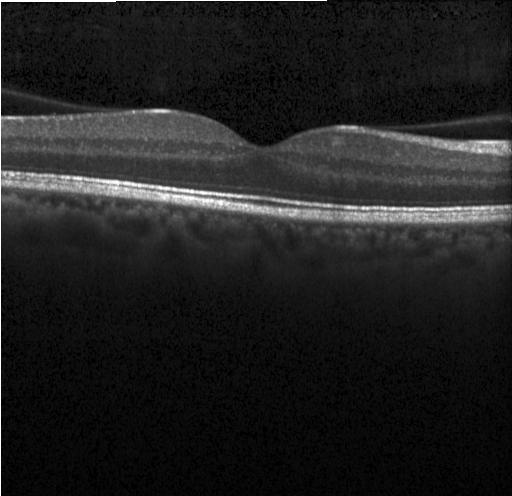
OCT finding: no CNV, no DME, and no drusen.